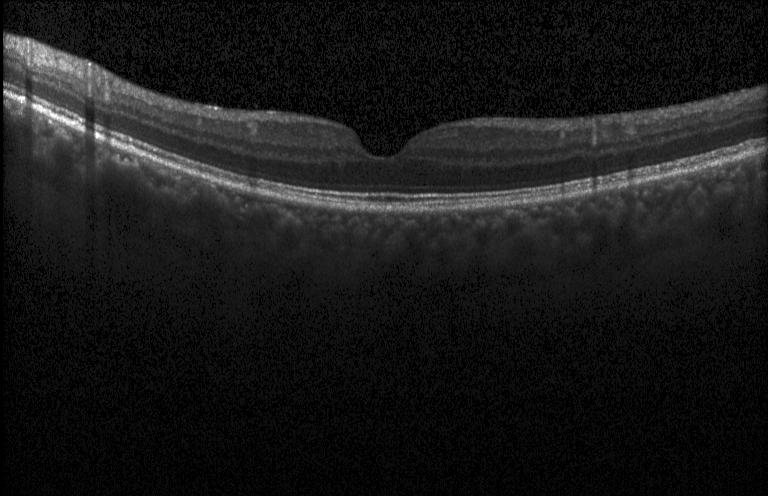
Macular OCT: no choroidal neovascularization, no diabetic macular edema, and no drusen.